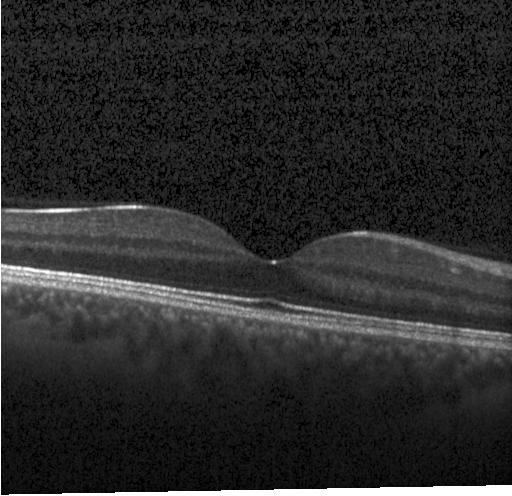
Diagnosis: no CNV, no DME, and no drusen.